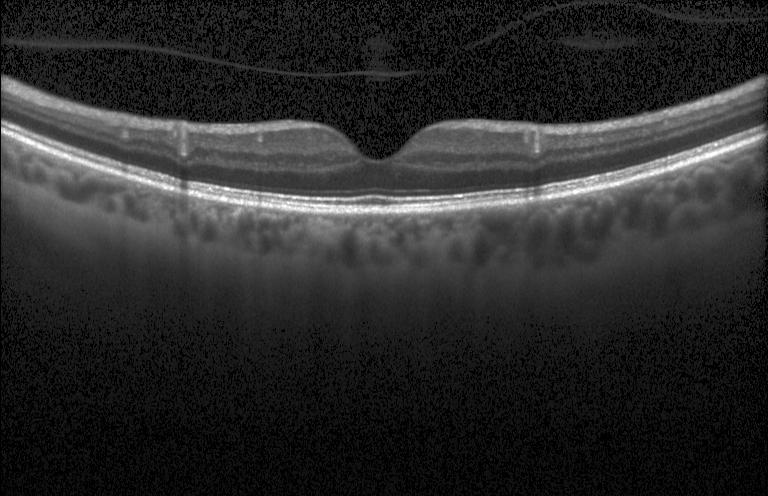 Spectral-domain optical coherence tomography. Optical coherence tomography B-scan. Macular scan. Acquired on a Heidelberg Spectralis — Assessment: no CNV, no DME, and no drusen.